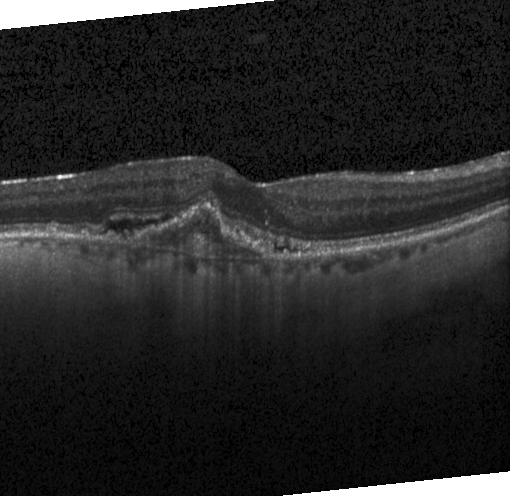
Dx: a choroidal neovascular membrane.